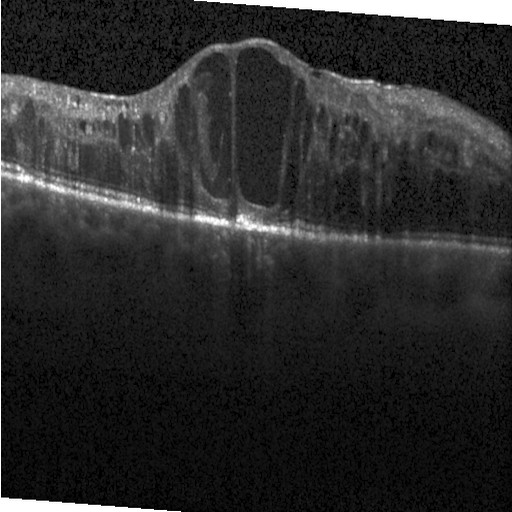
OCT B-scan — Diagnosis: diabetic macular edema.